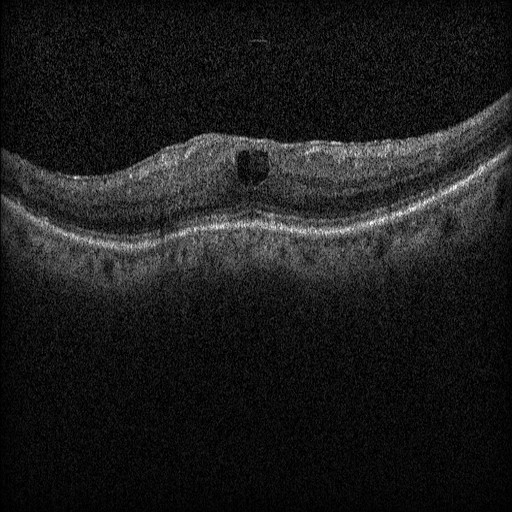

Optical coherence tomography B-scan — Diagnosis: diabetic macular edema.